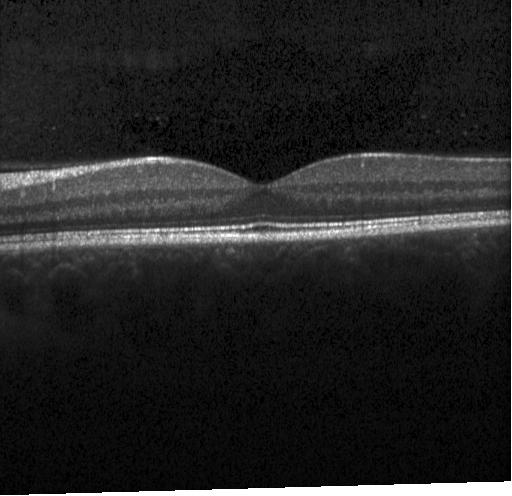

Dx: no choroidal neovascularization, no diabetic macular edema, and no drusen.